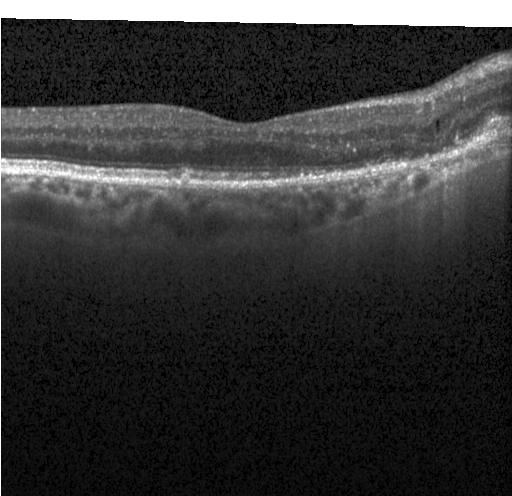
Macular OCT: a choroidal neovascular membrane.